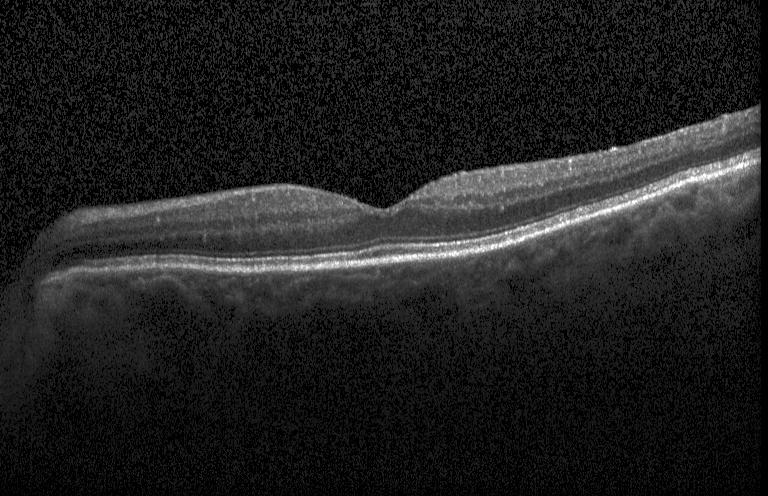
Finding: no choroidal neovascularization, diabetic macular edema, or drusen.